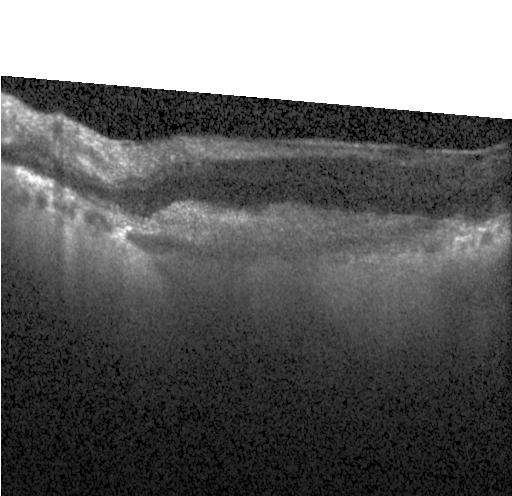 The scan shows choroidal neovascularization.